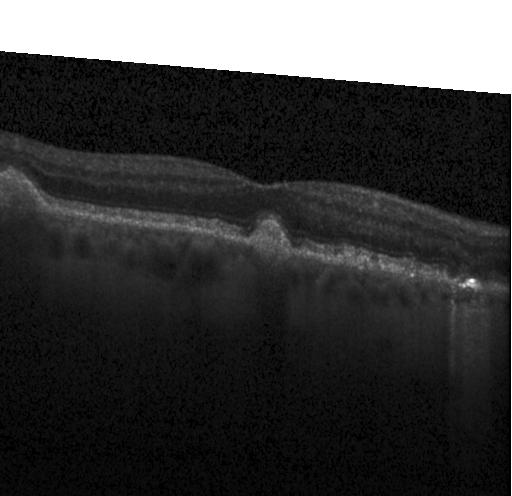
Finding: drusen.